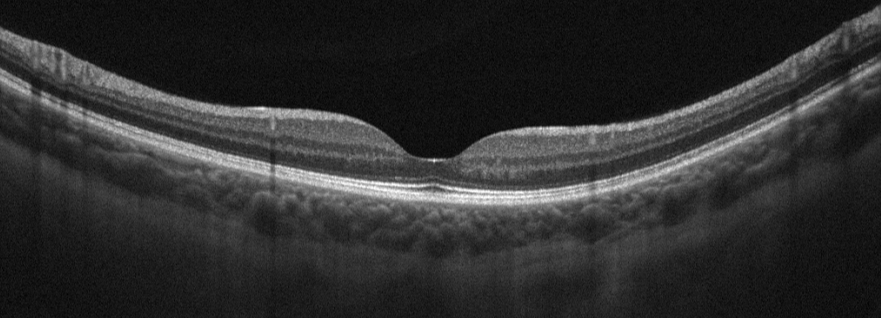
Retinal OCT cross-section. No AMD, DME, ERM, RAO, RVO, or VID.